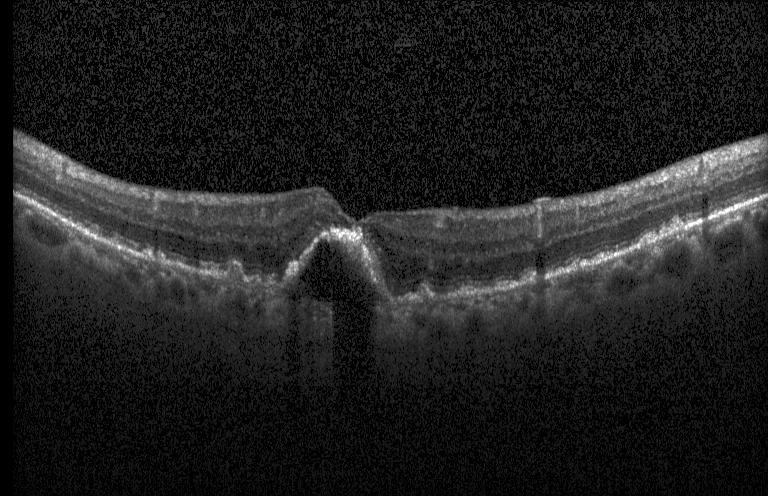 Acquired on a Heidelberg Spectralis. Retinal OCT cross-section. Centered on the fovea. Spectral-domain optical coherence tomography
Diagnosis: CNV.